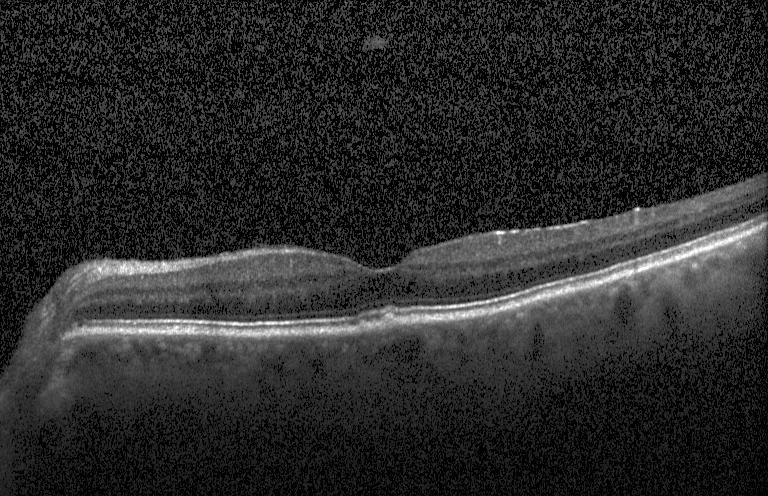 Optical coherence tomography B-scan · macular scan · spectral-domain optical coherence tomography · acquired on a Heidelberg Spectralis. Impression: multiple drusen.